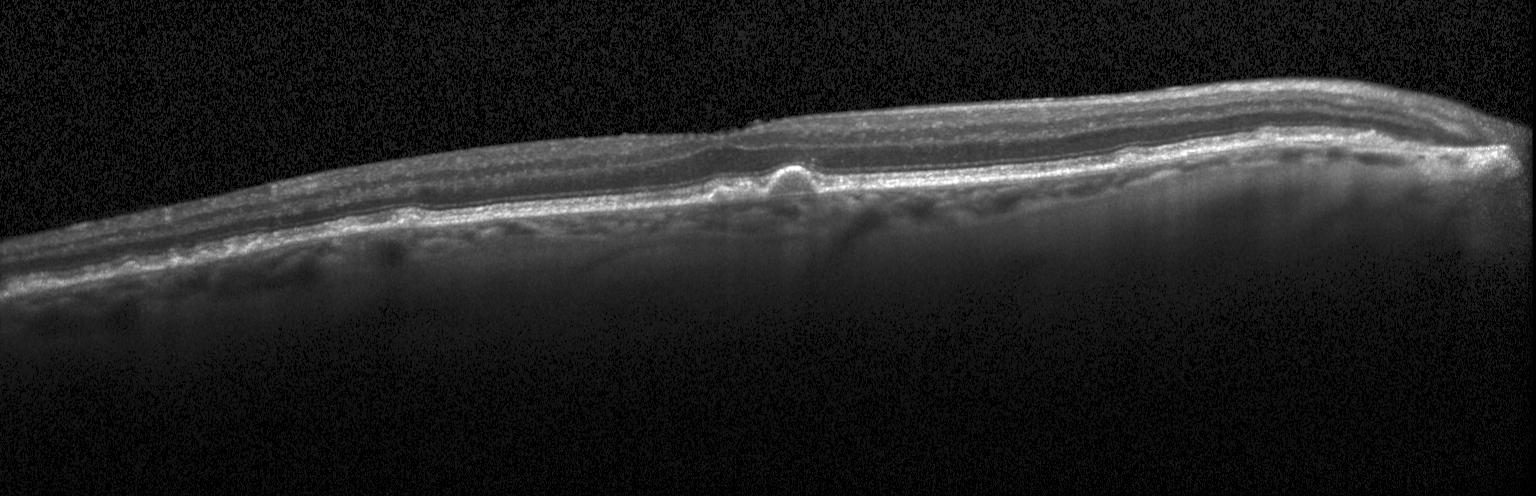
Optical coherence tomography B-scan; macular scan — Diagnosis: drusen.